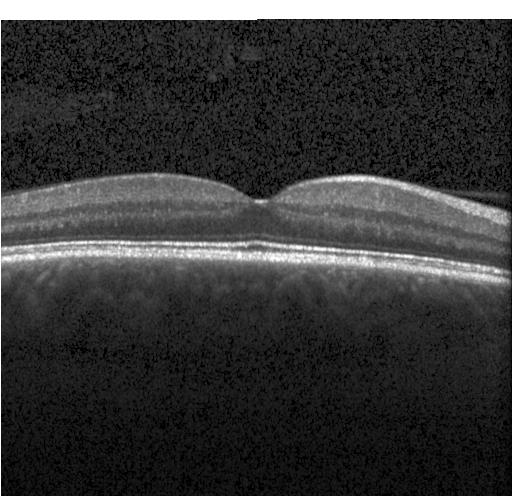

OCT line scan. Macular OCT: neither choroidal neovascularization, diabetic macular edema, nor drusen.